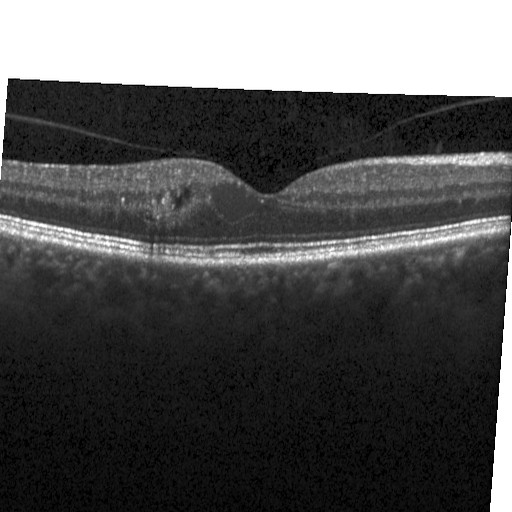
Impression: diabetic macular edema (DME).